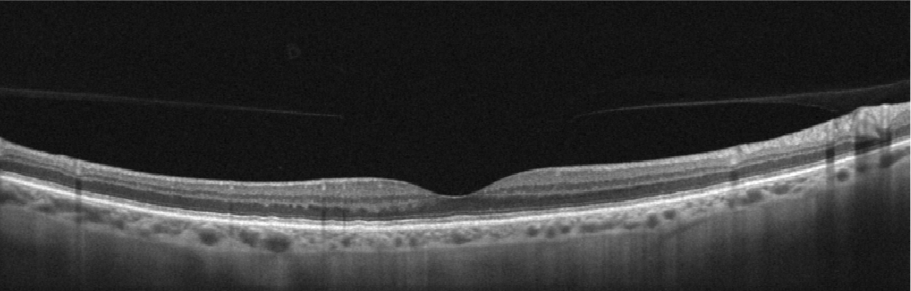

OCT B-scan
Assessment: age-related macular degeneration.